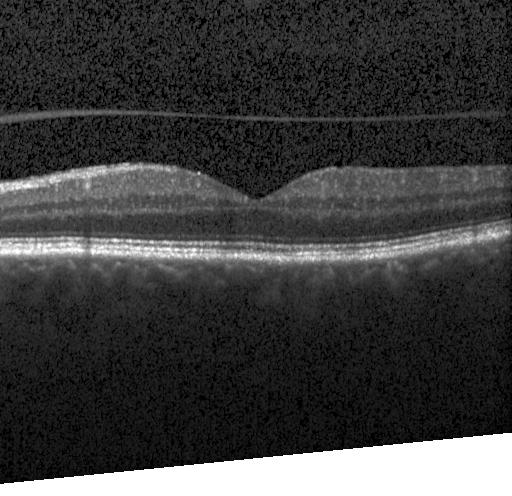
Spectral-domain OCT; OCT B-scan; centered on the fovea.
Finding: neither choroidal neovascularization, diabetic macular edema, nor drusen.